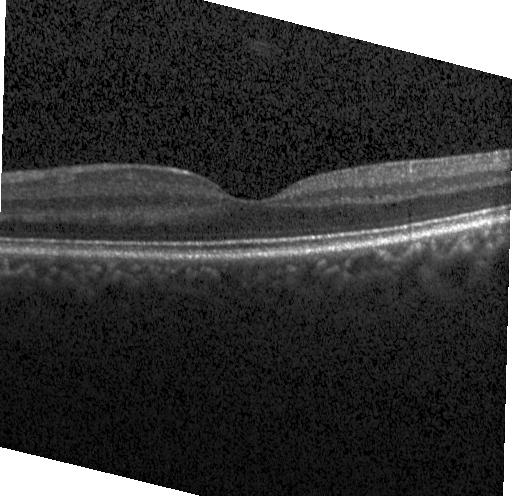
Impression: neither choroidal neovascularization, diabetic macular edema, nor drusen.